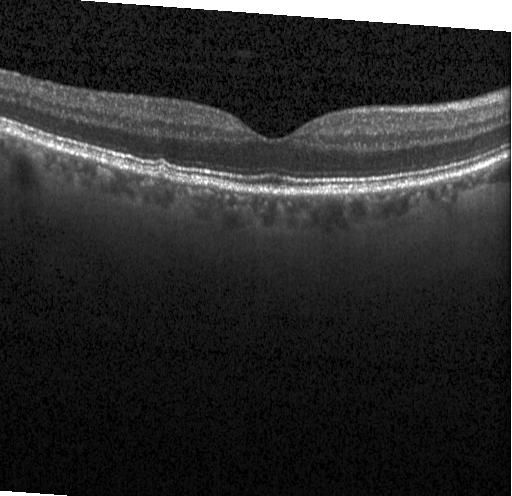
OCT B-scan, macular scan, SD-OCT, Heidelberg Spectralis
OCT finding: sub-RPE drusenoid deposits.